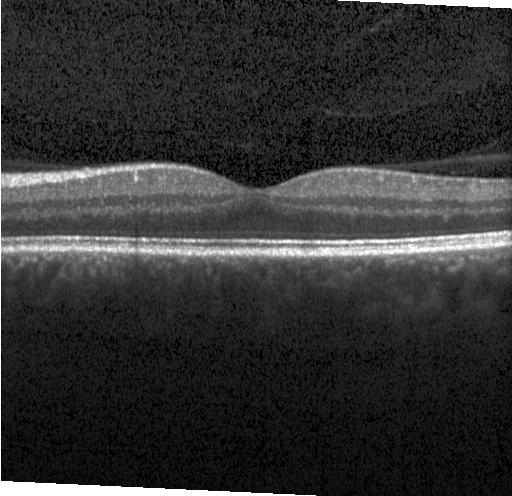 Retinal OCT cross-section showing no CNV, no DME, and no drusen.